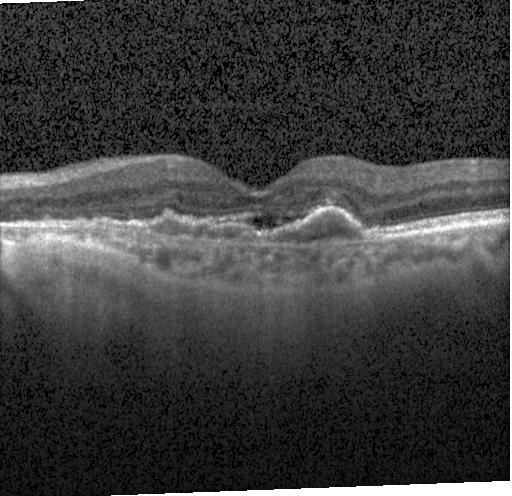 Optical coherence tomography scan. Fovea-centered.
Diagnosis: CNV.